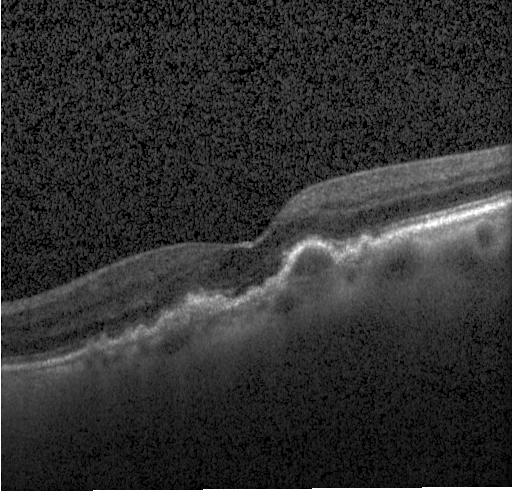
Finding: a choroidal neovascular membrane.